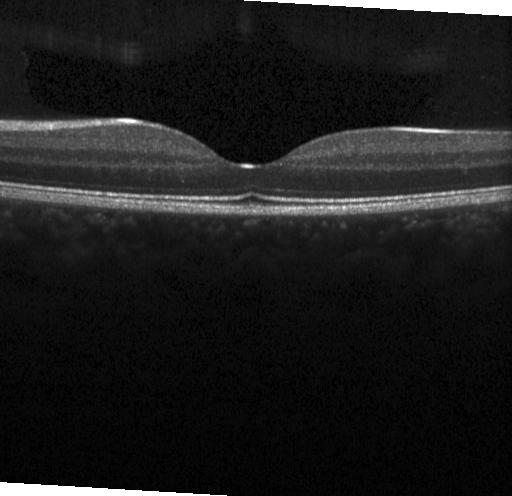
The scan shows no evidence of choroidal neovascularization, diabetic macular edema, or drusen.